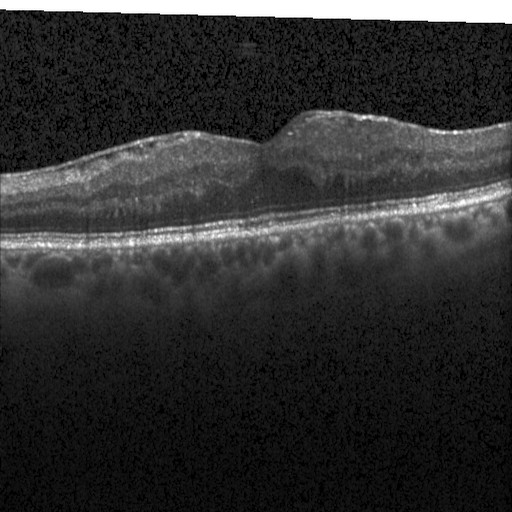

Macular OCT: diabetic macular edema.